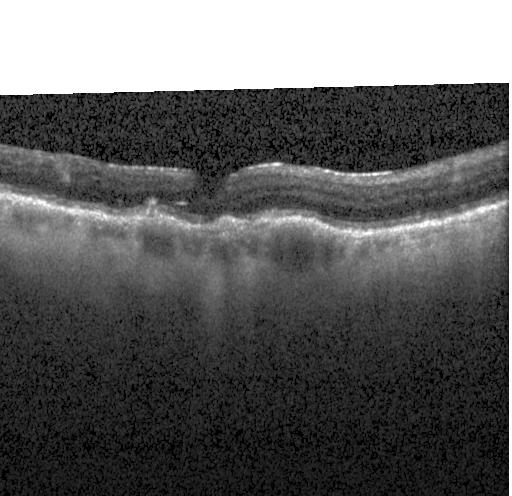
Retinal OCT B-scan · acquired on a Heidelberg Spectralis · spectral-domain OCT · fovea-centered — Dx: choroidal neovascularization (CNV).